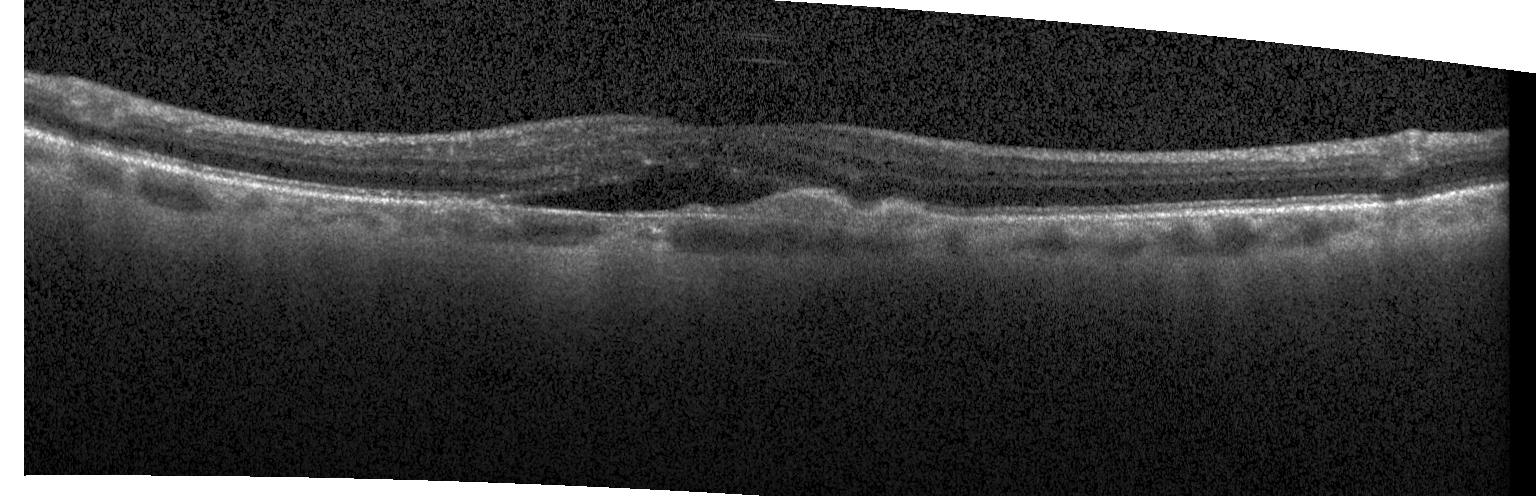

Impression: choroidal neovascularization (CNV).